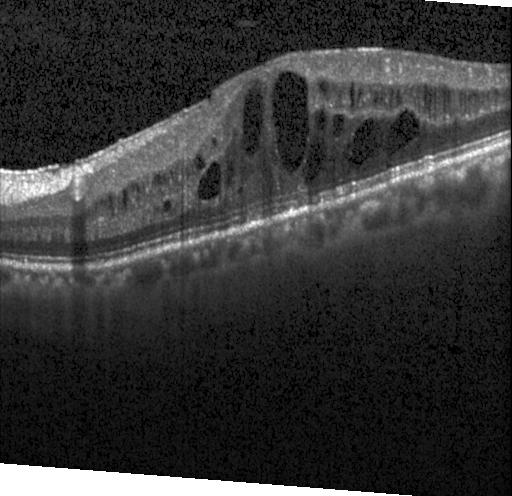

Spectral-domain optical coherence tomography, retinal OCT cross-section, horizontal scan through the fovea, Heidelberg Spectralis.
Finding: diabetic macular edema (DME).